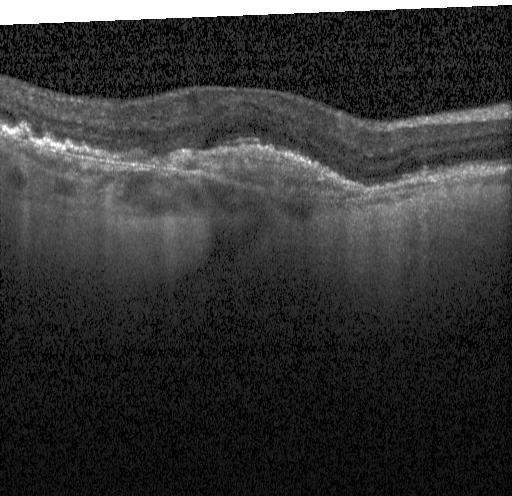
Assessment: CNV.